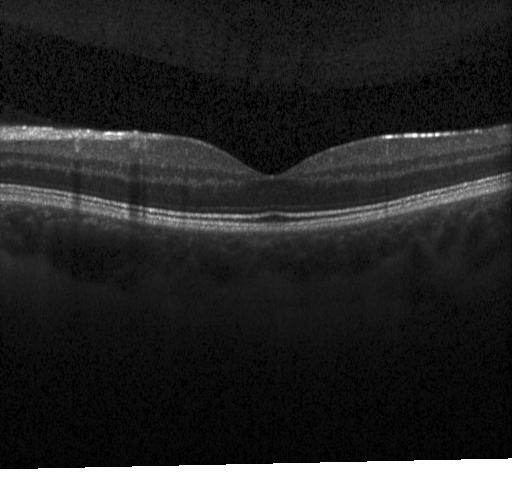

Spectral-domain OCT. Through the macula. Optical coherence tomography scan — Finding: no evidence of CNV, DME, or drusen.